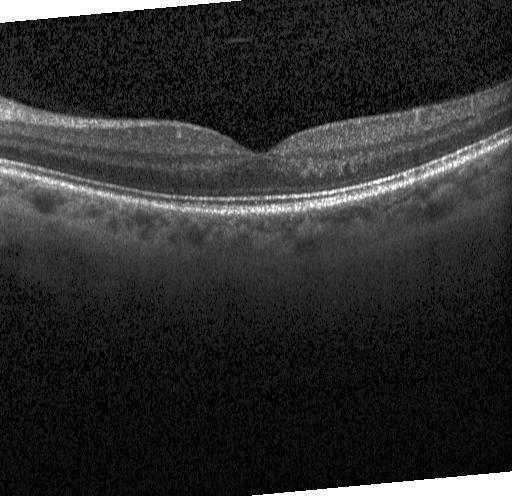 OCT B-scan · instrument: Heidelberg Spectralis. Diagnosis: neither CNV, DME, nor drusen.